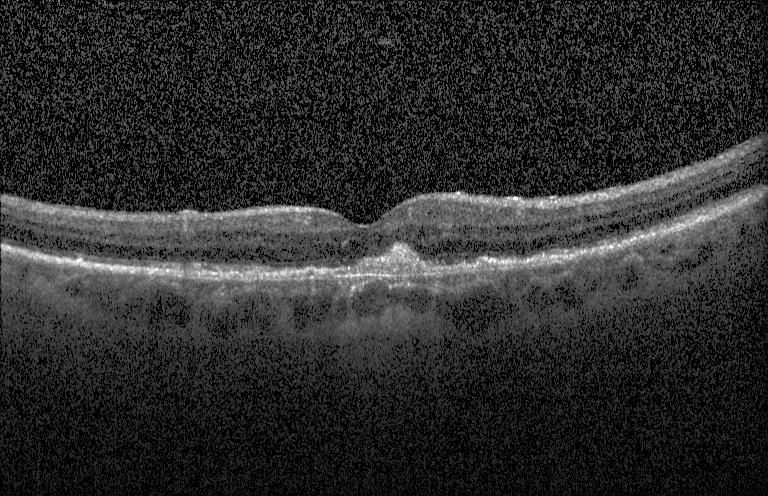 OCT line scan · through the macula.
Dx: a choroidal neovascular membrane.